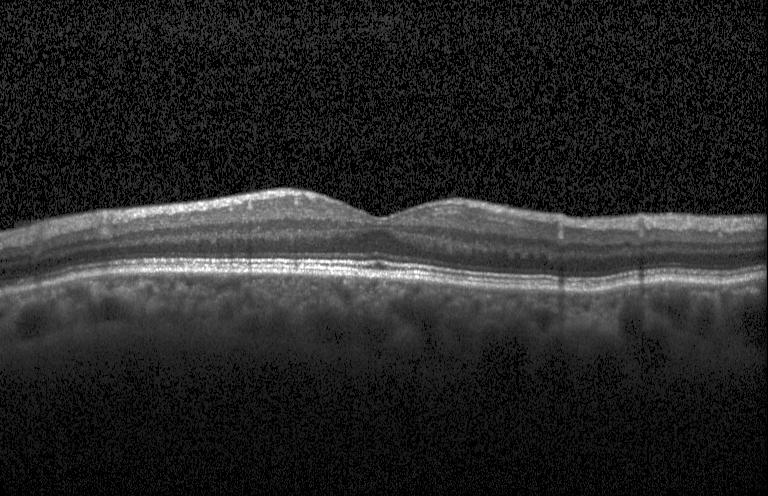

Dx: no choroidal neovascularization, diabetic macular edema, or drusen.